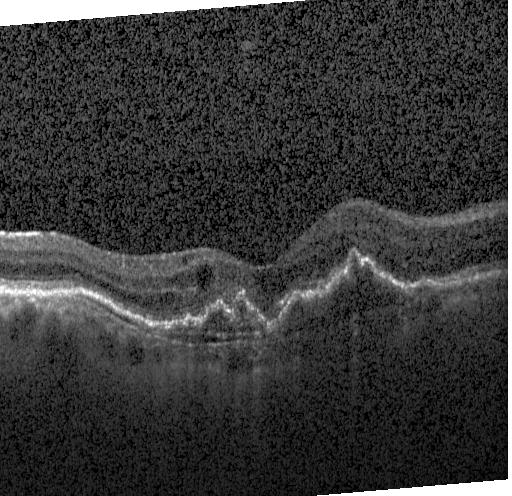

OCT finding: a choroidal neovascular membrane.